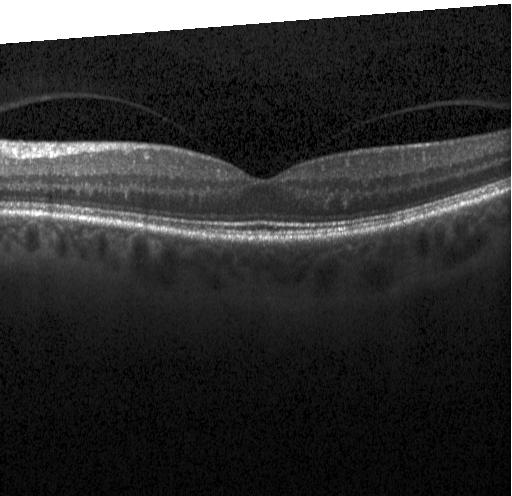 Spectral-domain optical coherence tomography; through the macula; Heidelberg Spectralis; OCT line scan.
Finding: neither choroidal neovascularization, diabetic macular edema, nor drusen.